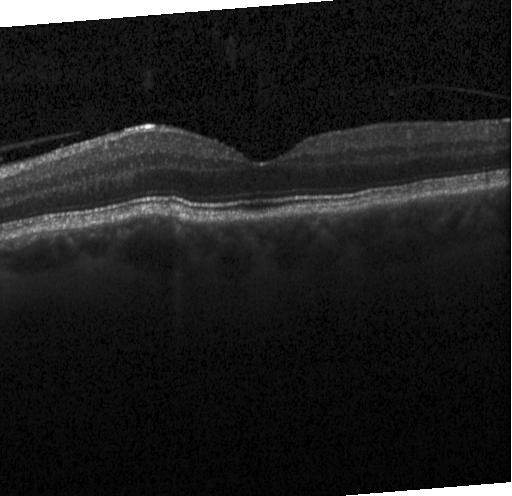
Optical coherence tomography scan; horizontal scan through the fovea.
Finding: no choroidal neovascularization, no diabetic macular edema, and no drusen.